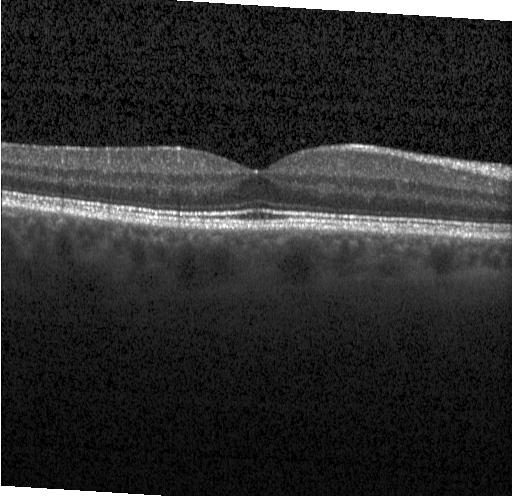

OCT finding: no evidence of CNV, DME, or drusen.